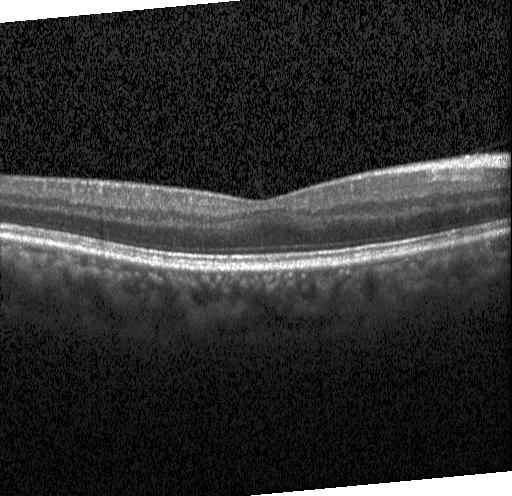

Impression: no evidence of choroidal neovascularization, diabetic macular edema, or drusen.